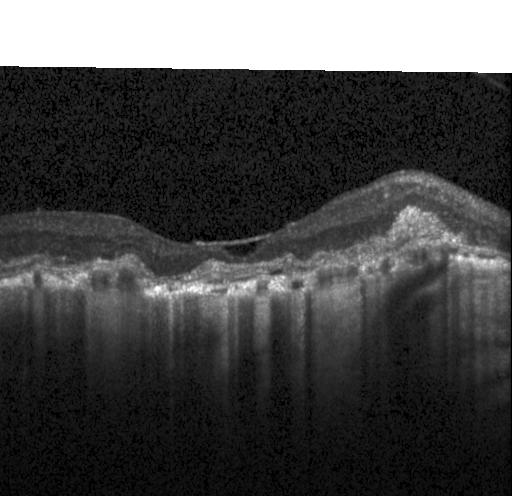
Macular OCT: CNV.